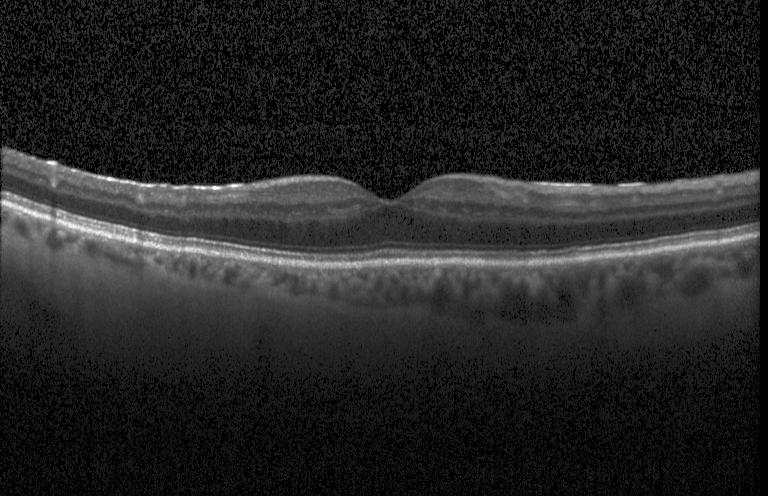

Macular OCT: no CNV, DME, or drusen.